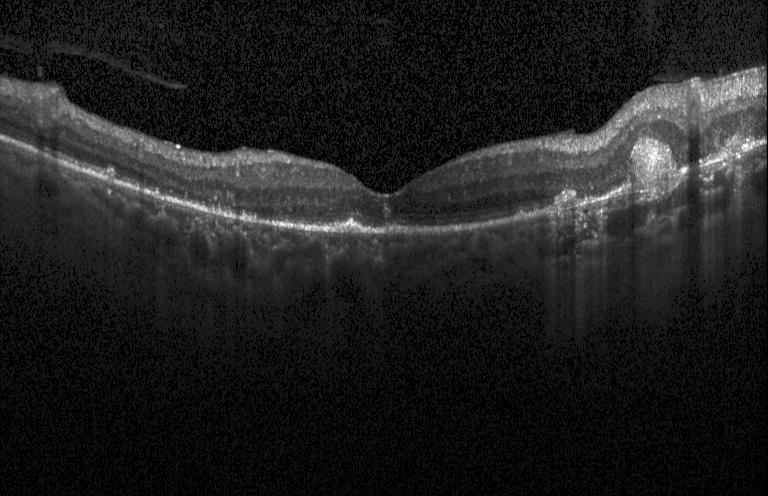 Macular OCT demonstrating CNV.